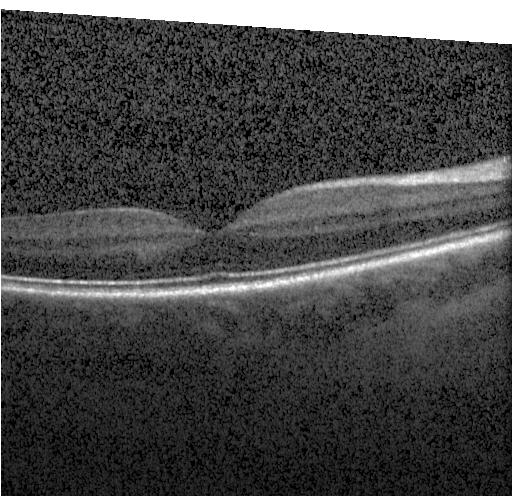

Finding: no choroidal neovascularization, diabetic macular edema, or drusen.